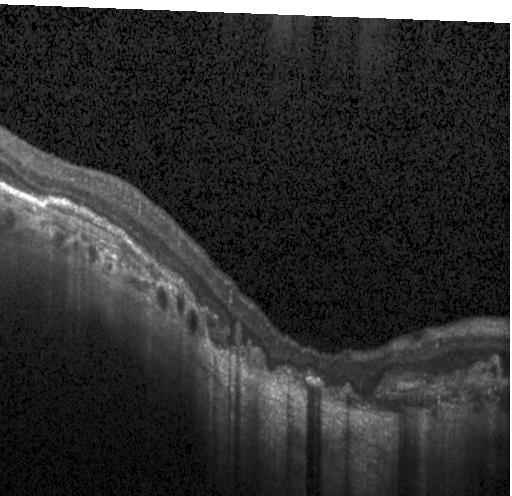
Retinal OCT B-scan; horizontal scan through the fovea; spectral-domain optical coherence tomography; instrument: Heidelberg Spectralis.
OCT finding: choroidal neovascularization.